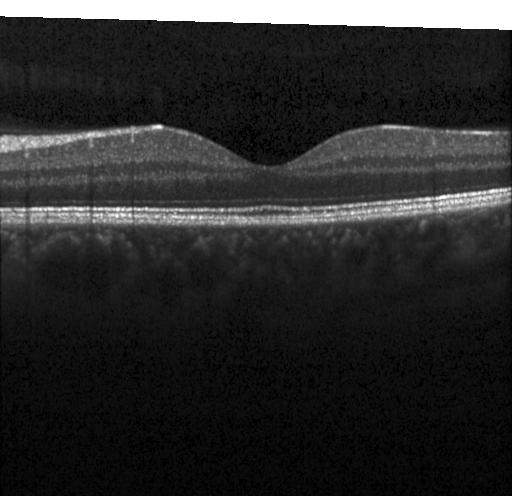 Retinal OCT cross-section — Finding: no CNV, no DME, and no drusen.